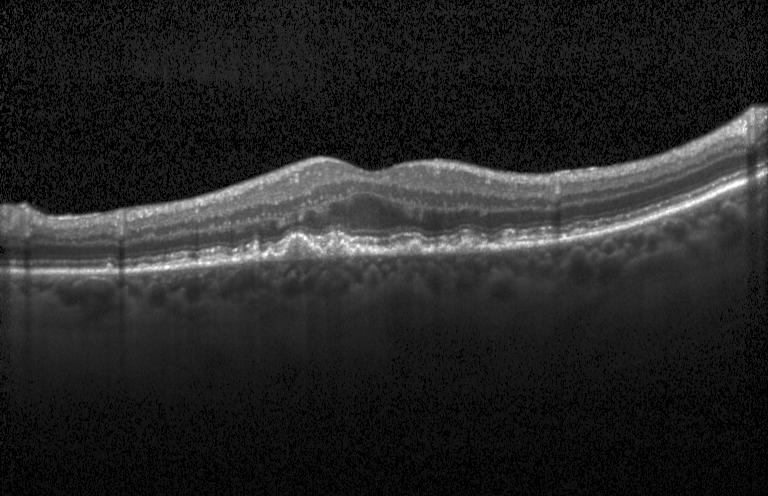 Assessment: multiple drusen.